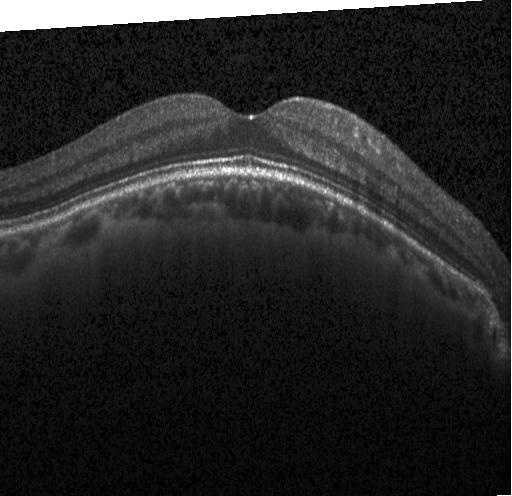
Spectral-domain optical coherence tomography · retinal OCT B-scan · Heidelberg Spectralis OCT system.
The scan shows no CNV, no DME, and no drusen.